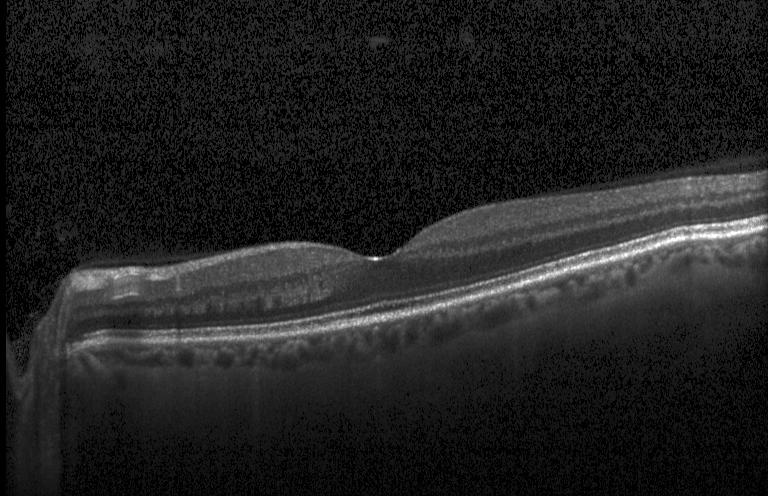
Retinal OCT cross-section showing no CNV, no DME, and no drusen.